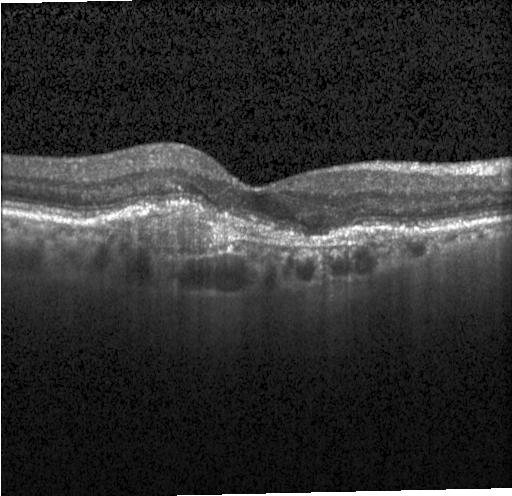

Retinal OCT B-scan; macular scan
OCT finding: a choroidal neovascular membrane.